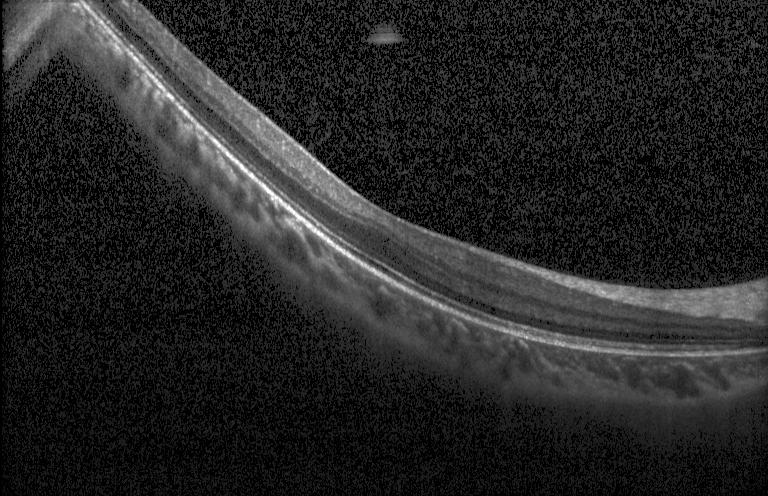

Retinal OCT B-scan. Diagnosis: no evidence of choroidal neovascularization, diabetic macular edema, or drusen.